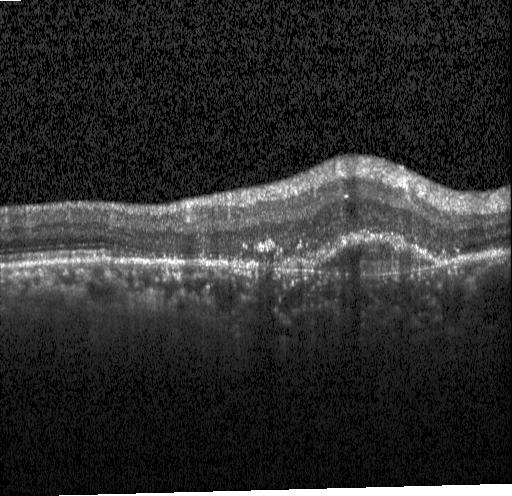 Macular OCT demonstrating CNV.